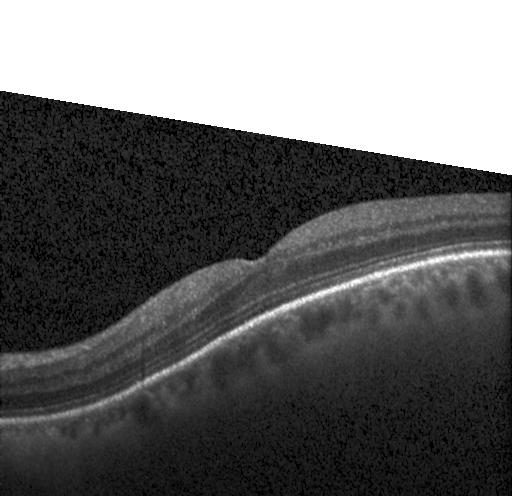

Finding: neither choroidal neovascularization, diabetic macular edema, nor drusen.